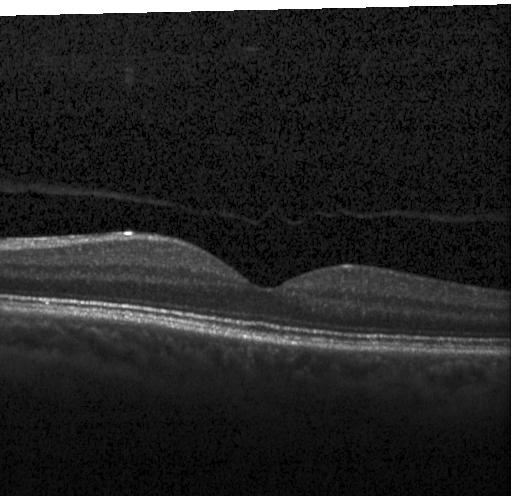
Optical coherence tomography scan; acquired on a Heidelberg Spectralis; spectral-domain optical coherence tomography; centered on the fovea — The scan shows no evidence of choroidal neovascularization, diabetic macular edema, or drusen.